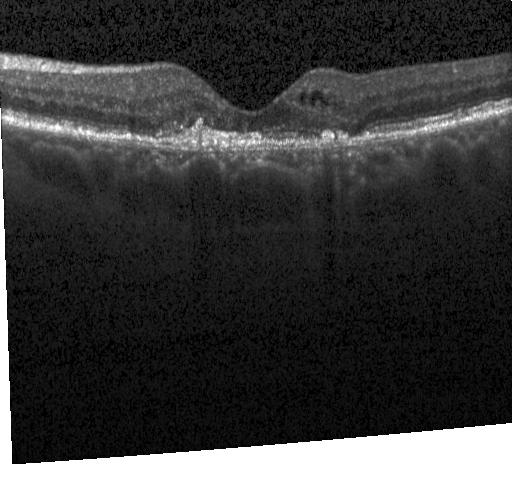
Optical coherence tomography B-scan. SD-OCT. Through the macula. Instrument: Heidelberg Spectralis. Diagnosis: choroidal neovascularization (CNV).